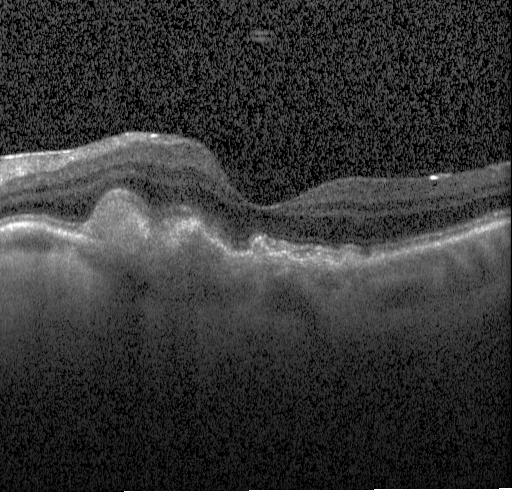

Spectral-domain OCT. Retinal OCT B-scan. Heidelberg Spectralis. Through the macula. Assessment: choroidal neovascularization (CNV).